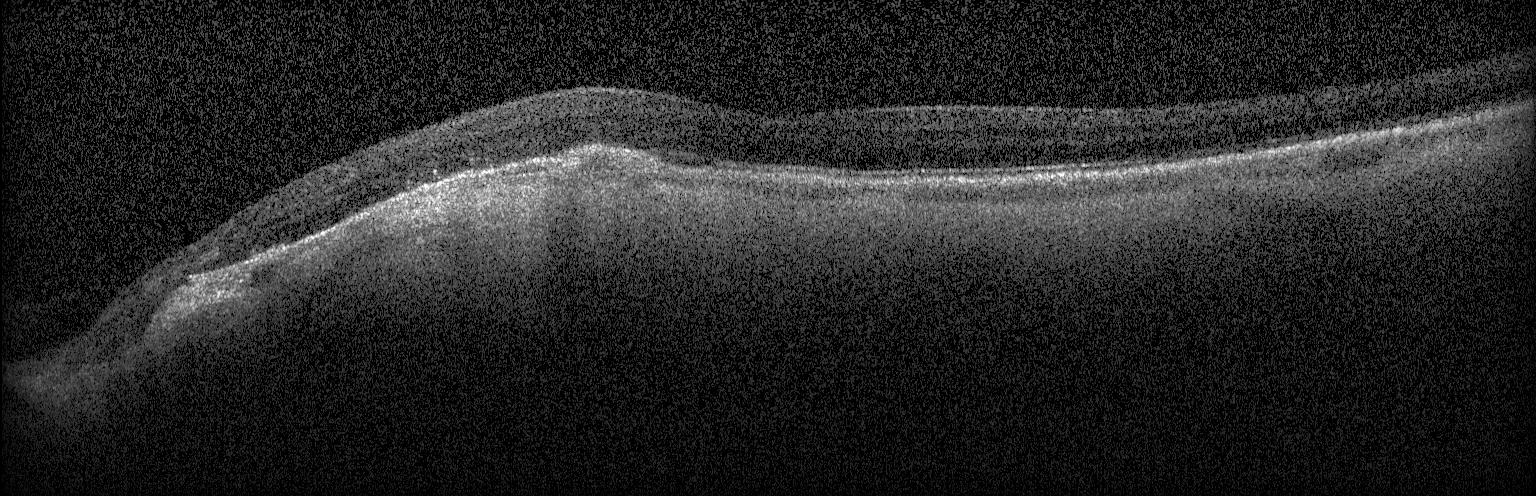
OCT line scan, Heidelberg Spectralis
The scan shows a choroidal neovascular membrane.